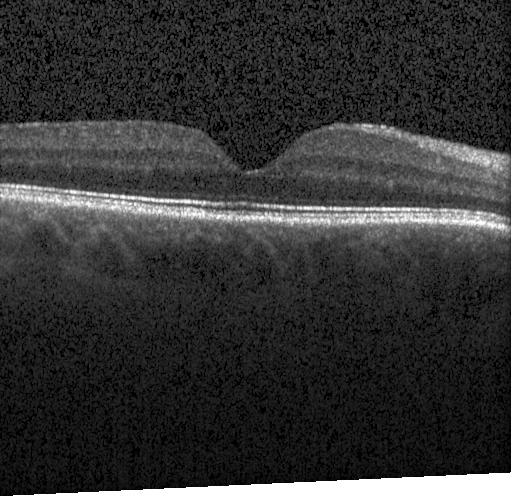 Finding: neither choroidal neovascularization, diabetic macular edema, nor drusen.